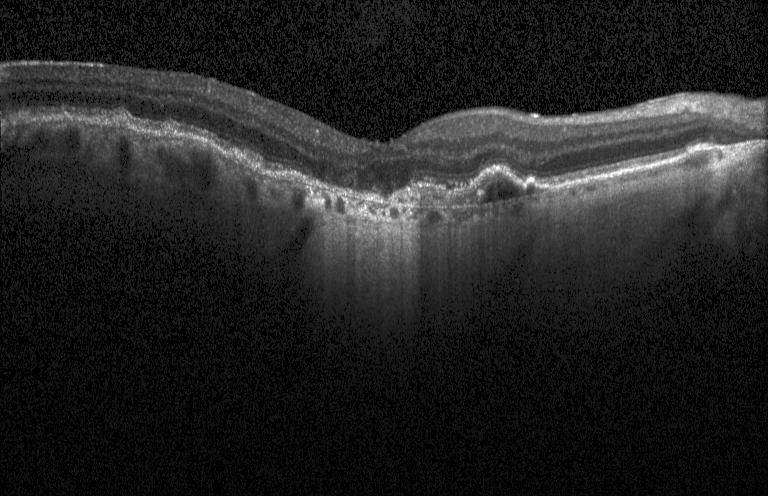

Optical coherence tomography scan.
OCT finding: CNV.